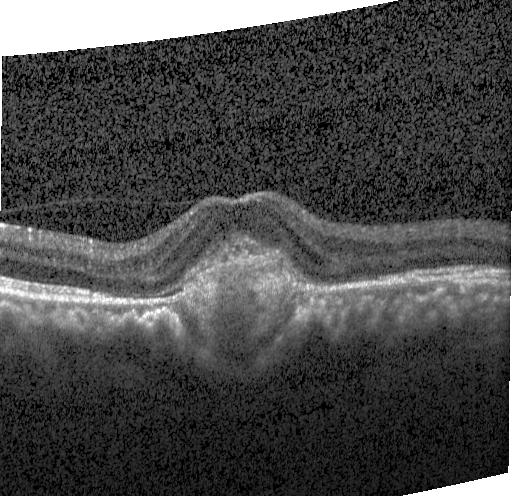
OCT line scan, acquired on a Heidelberg Spectralis, centered on the fovea — OCT finding: CNV.